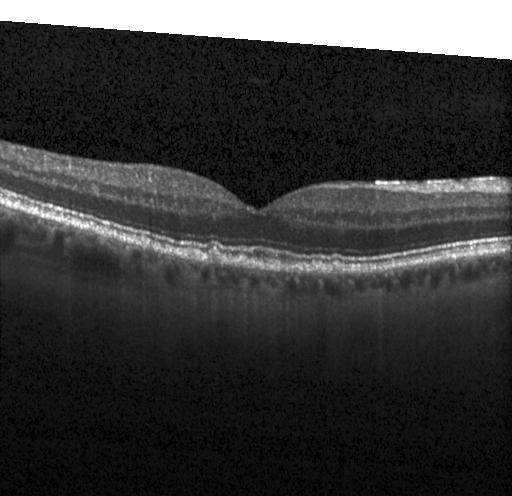

The scan shows multiple drusen.